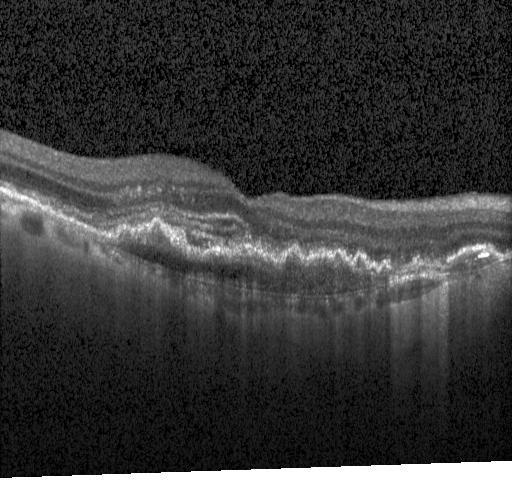 Optical coherence tomography scan. SD-OCT. Instrument: Heidelberg Spectralis.
This B-scan demonstrates choroidal neovascularization.